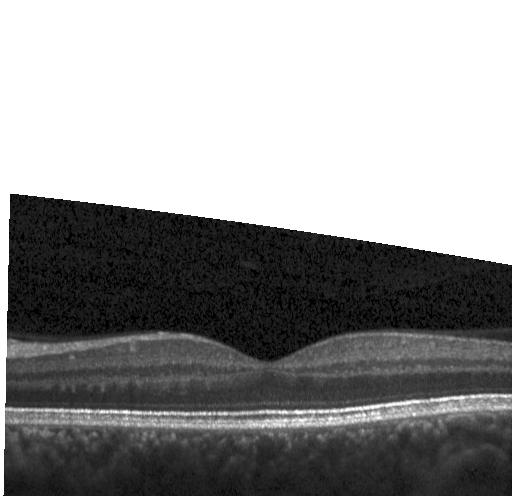

This B-scan demonstrates no choroidal neovascularization, diabetic macular edema, or drusen.